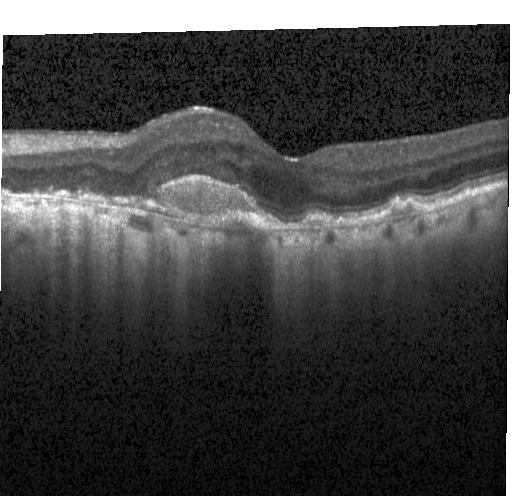
OCT finding: a choroidal neovascular membrane.